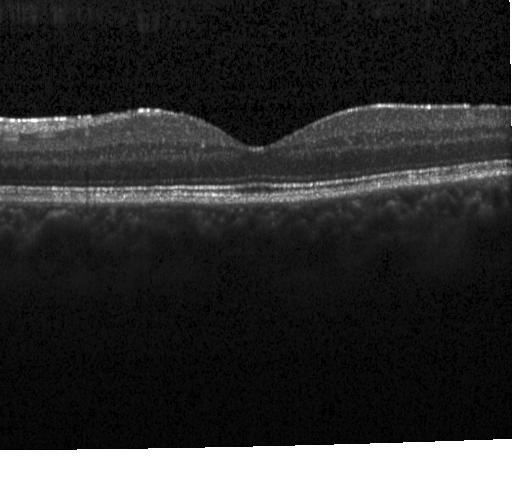 Optical coherence tomography scan. Centered on the fovea
Macular OCT: no choroidal neovascularization, diabetic macular edema, or drusen.